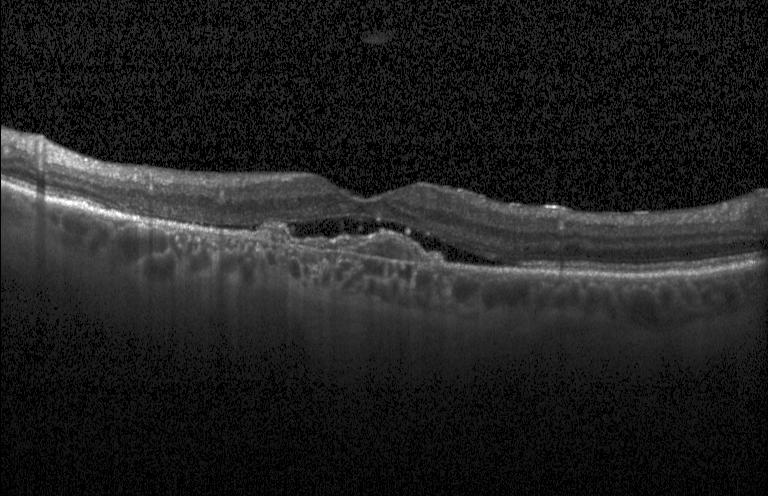 OCT finding: choroidal neovascularization.